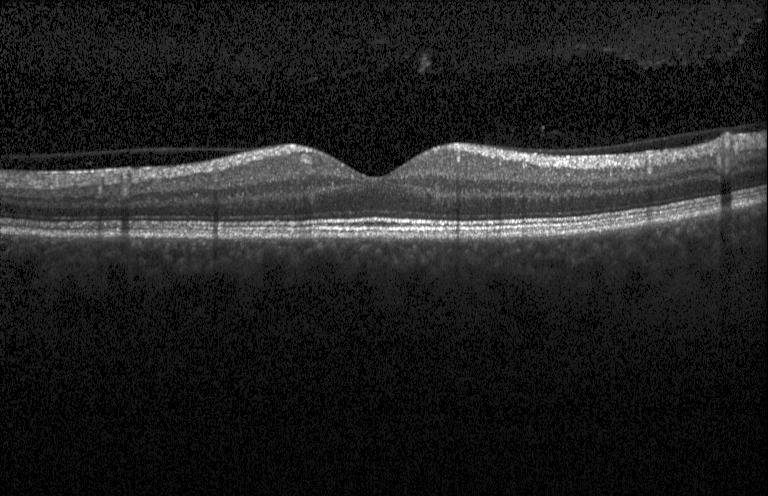 Optical coherence tomography B-scan.
OCT finding: neither choroidal neovascularization, diabetic macular edema, nor drusen.